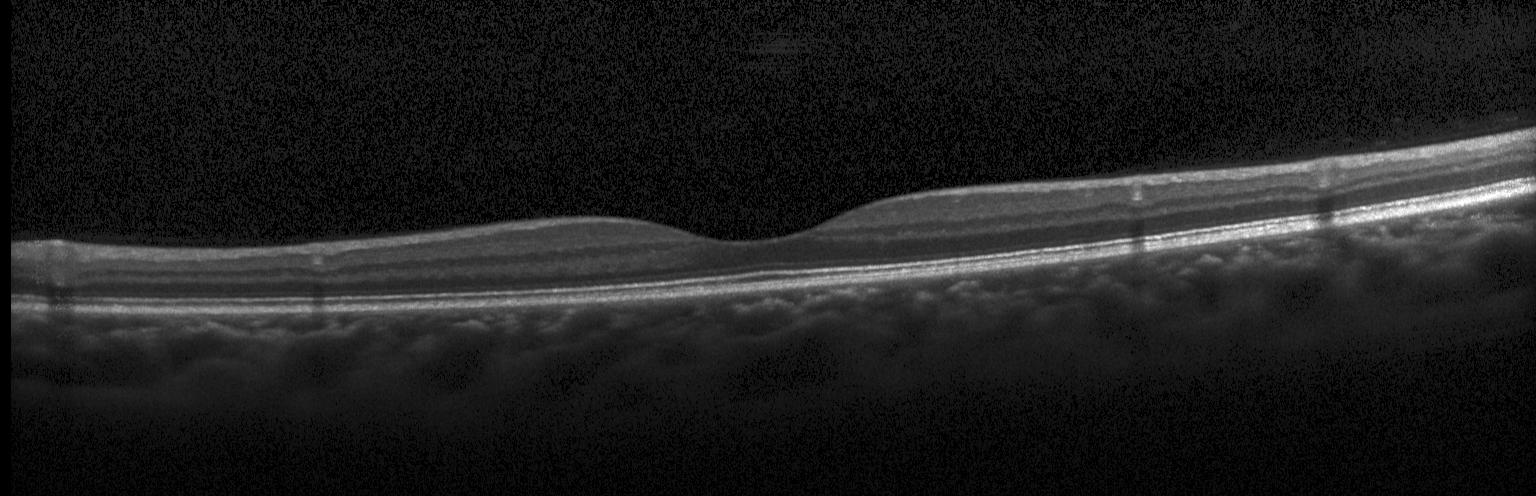

Retinal OCT B-scan, macular scan, Heidelberg Spectralis OCT system — This B-scan demonstrates no evidence of CNV, DME, or drusen.